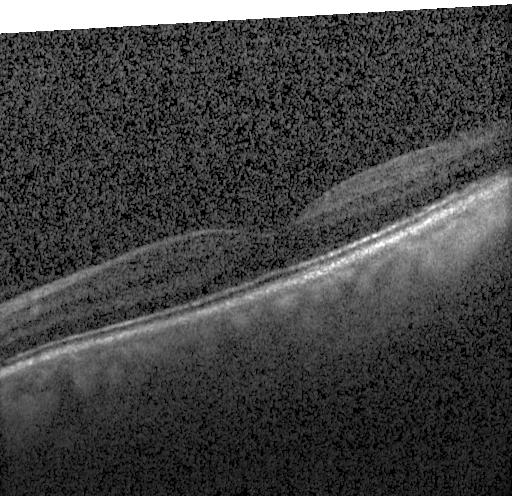 Assessment: neither choroidal neovascularization, diabetic macular edema, nor drusen.